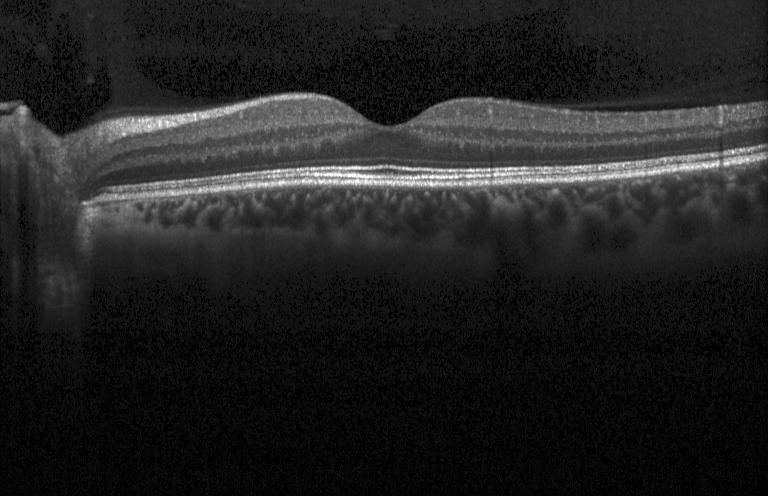
The scan shows neither choroidal neovascularization, diabetic macular edema, nor drusen.